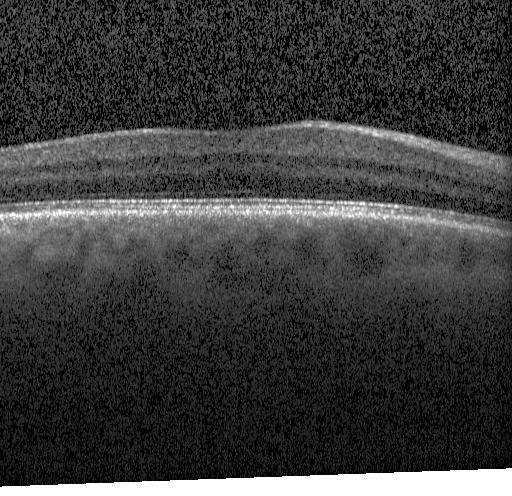 OCT line scan
Neither choroidal neovascularization, diabetic macular edema, nor drusen.